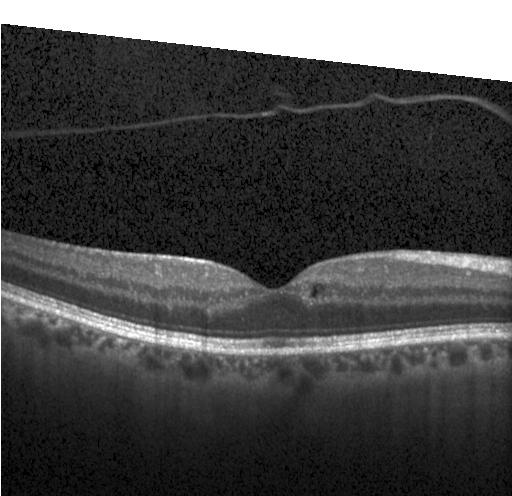 Acquired on a Heidelberg Spectralis · optical coherence tomography scan · spectral-domain optical coherence tomography · fovea-centered — This B-scan demonstrates diabetic macular edema (DME).